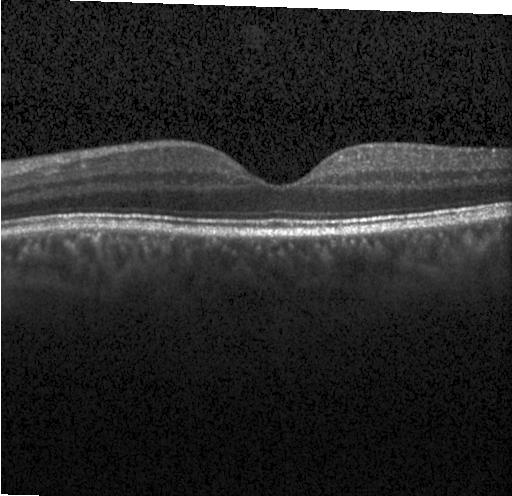 Dx: neither CNV, DME, nor drusen.